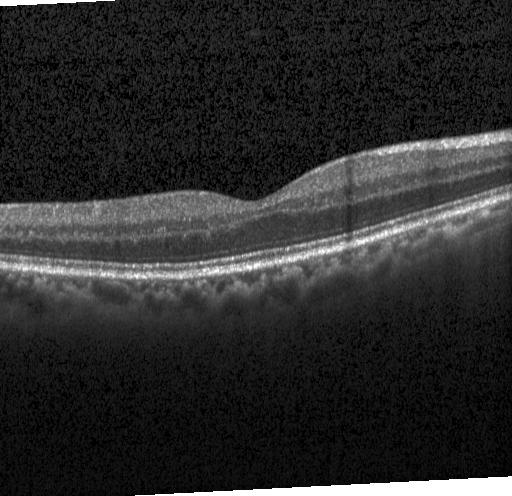 Retinal OCT B-scan. OCT finding: no evidence of choroidal neovascularization, diabetic macular edema, or drusen.